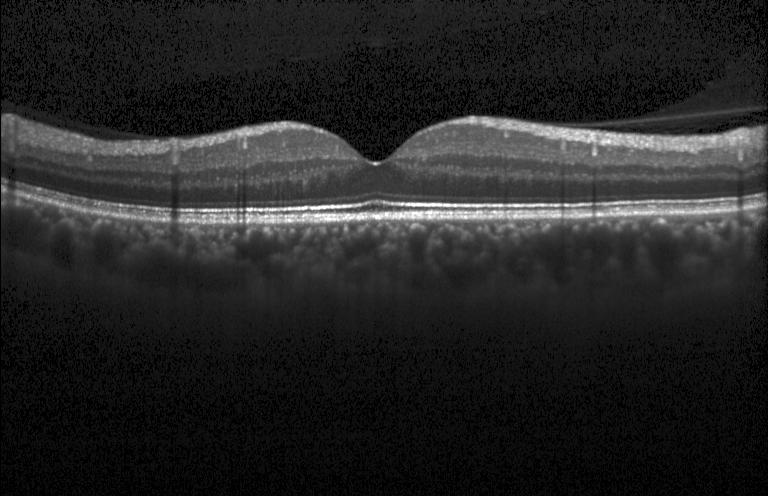
OCT line scan
Impression: no evidence of choroidal neovascularization, diabetic macular edema, or drusen.